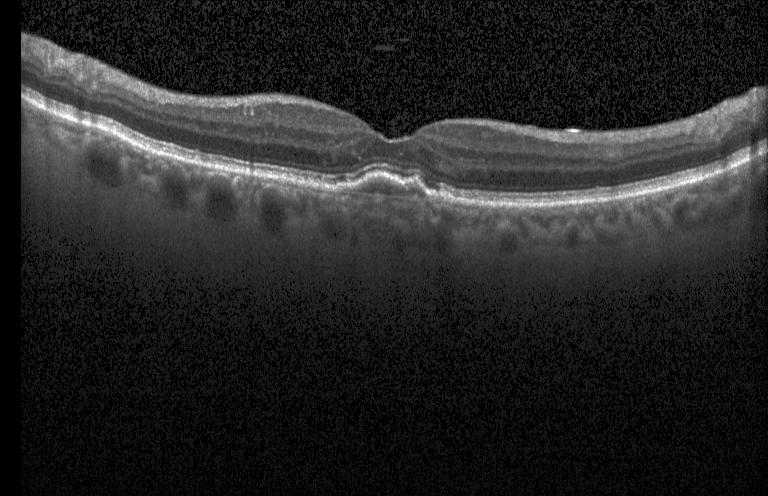

OCT finding: a choroidal neovascular membrane.